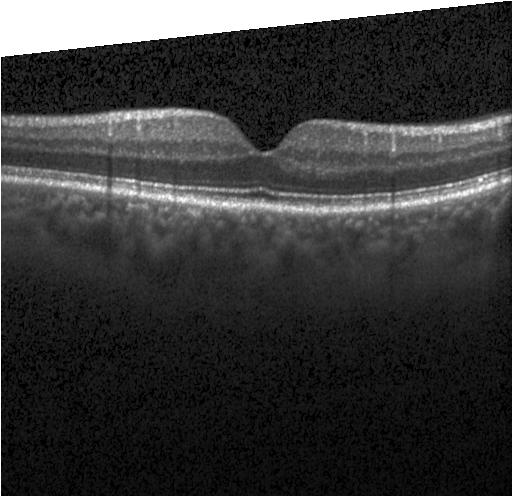

Optical coherence tomography B-scan. Instrument: Heidelberg Spectralis. The scan shows no evidence of choroidal neovascularization, diabetic macular edema, or drusen.